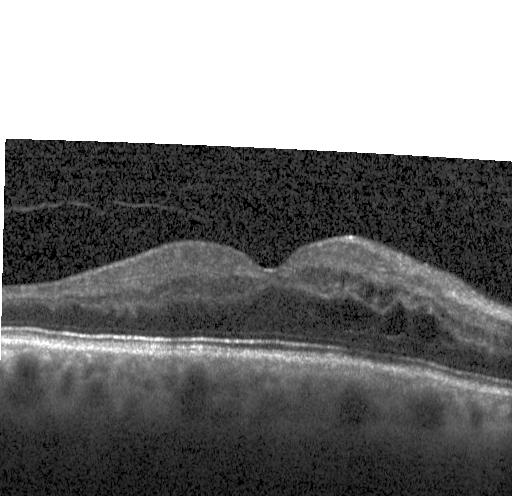 Finding: DME.